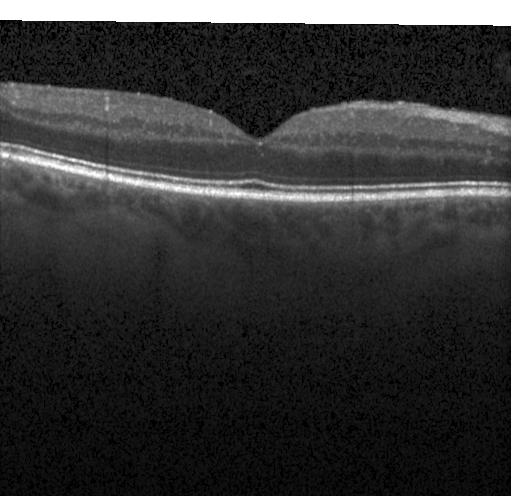

OCT B-scan. The scan shows no evidence of choroidal neovascularization, diabetic macular edema, or drusen.